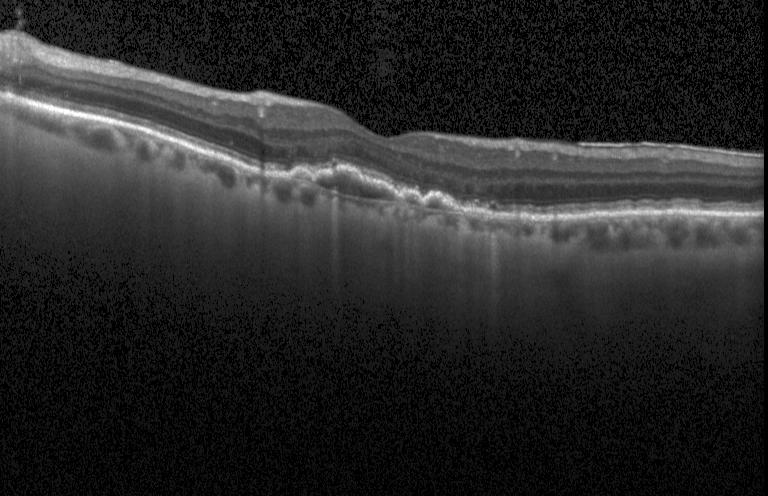

OCT finding: a choroidal neovascular membrane.